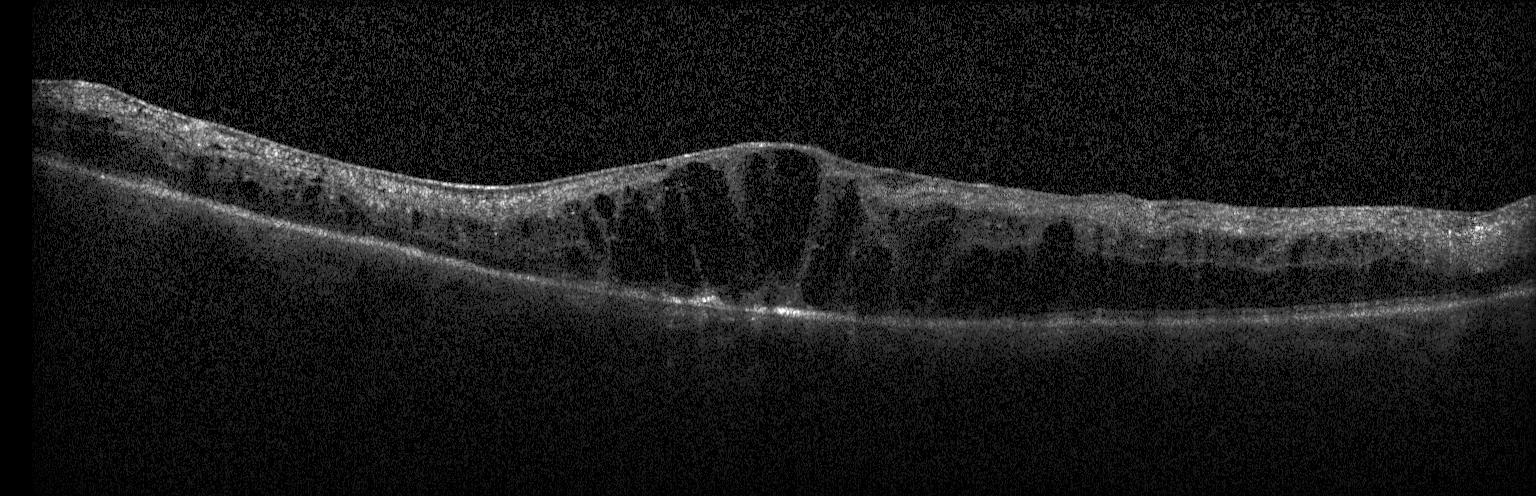 Spectral-domain OCT, Heidelberg Spectralis OCT system, centered on the fovea, optical coherence tomography B-scan
OCT finding: diabetic macular edema (DME).